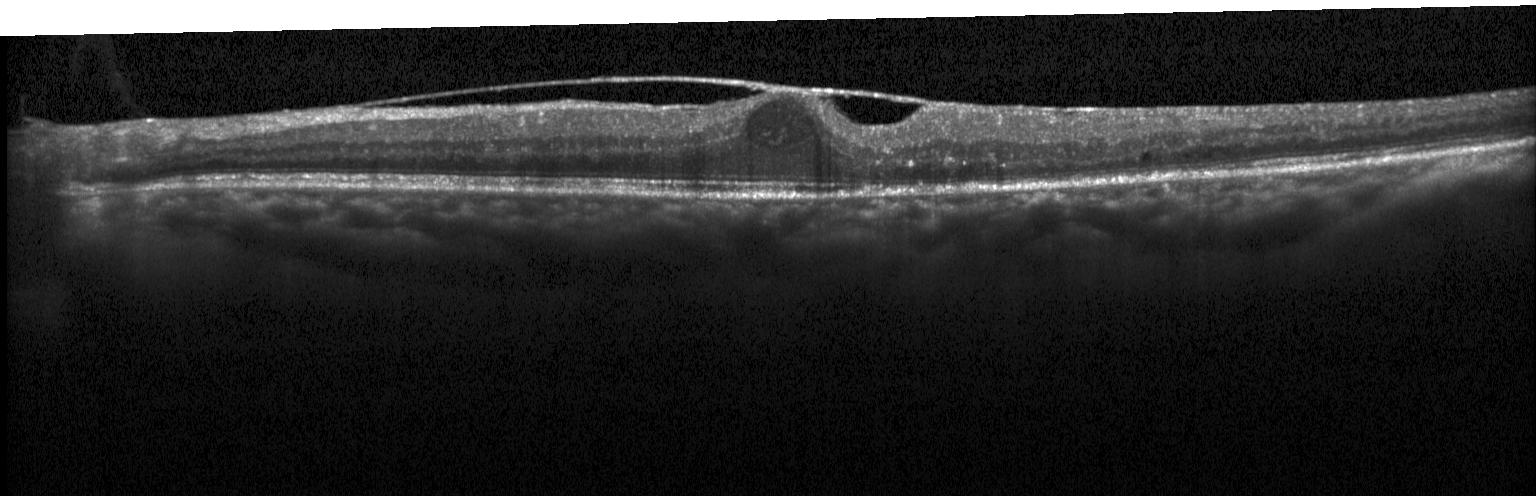

Spectral-domain OCT · instrument: Heidelberg Spectralis · horizontal scan through the fovea · retinal OCT B-scan
OCT finding: diabetic macular edema (DME).